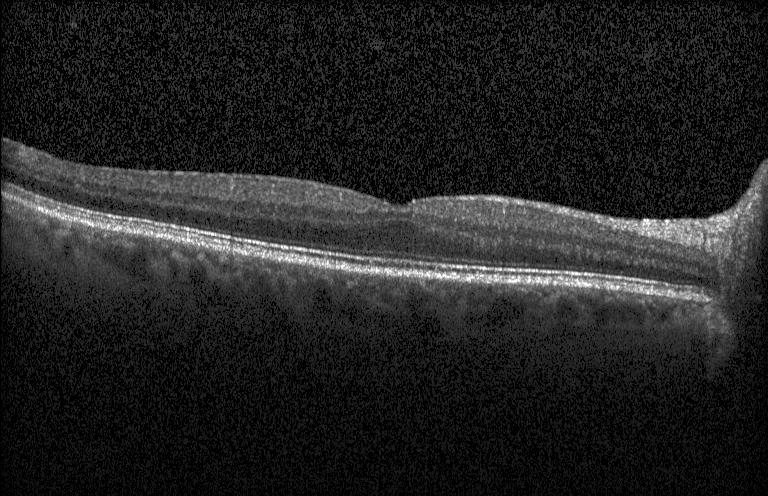

Retinal OCT B-scan. Through the macula. SD-OCT.
Assessment: no CNV, no DME, and no drusen.